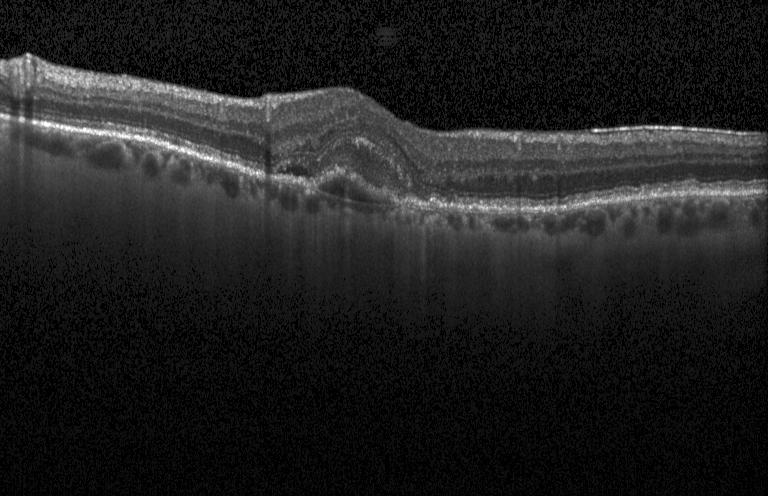 Retinal OCT B-scan, SD-OCT, centered on the fovea.
Diagnosis: a choroidal neovascular membrane.